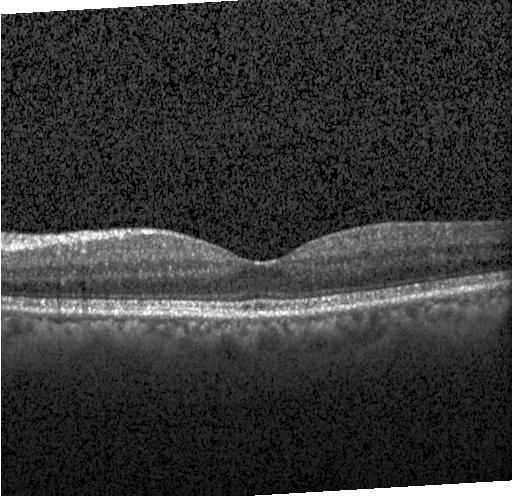
Macular OCT demonstrating no evidence of CNV, DME, or drusen.